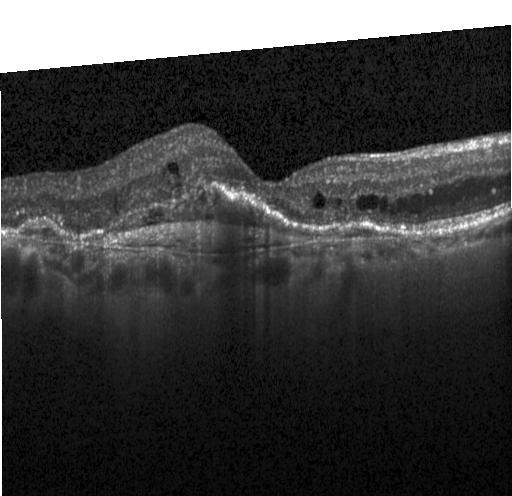 Optical coherence tomography scan · acquired on a Heidelberg Spectralis · horizontal scan through the fovea. Finding: choroidal neovascularization.